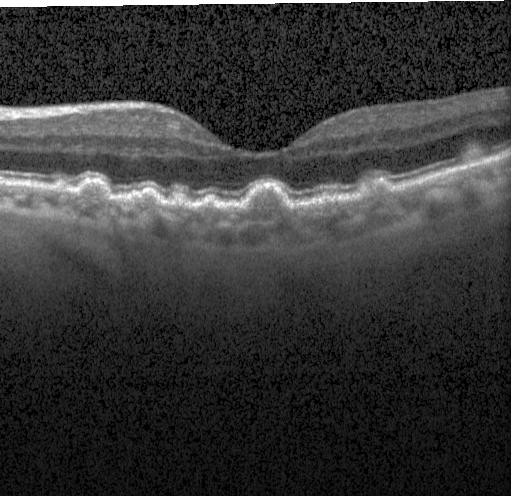 Optical coherence tomography scan, acquired on a Heidelberg Spectralis, spectral-domain optical coherence tomography, macular scan.
The scan shows multiple drusen.